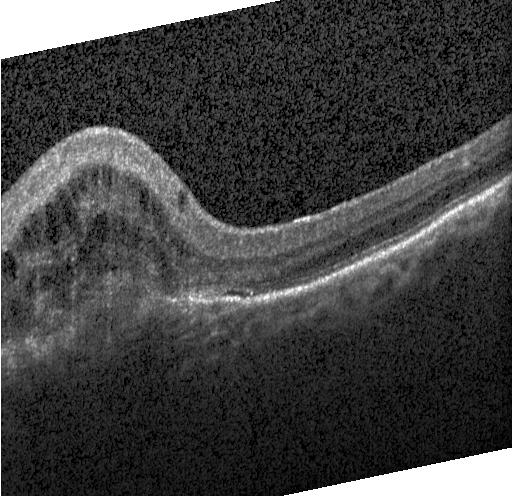

Heidelberg Spectralis; fovea-centered; spectral-domain OCT; retinal OCT cross-section. A choroidal neovascular membrane.